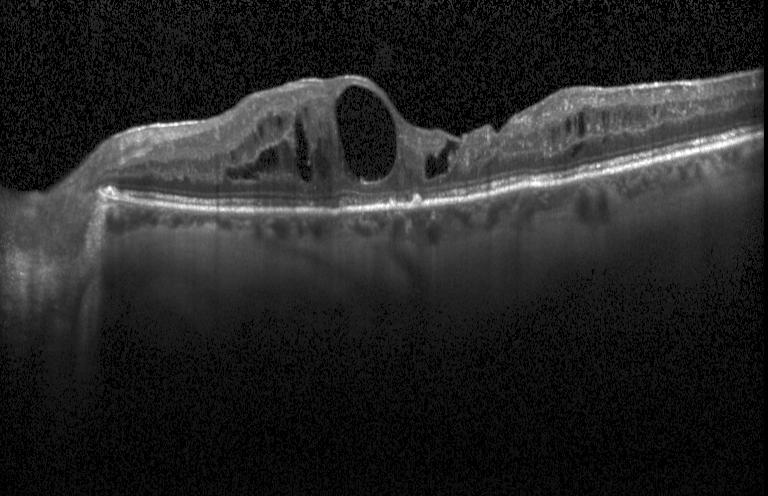 Impression: DME.